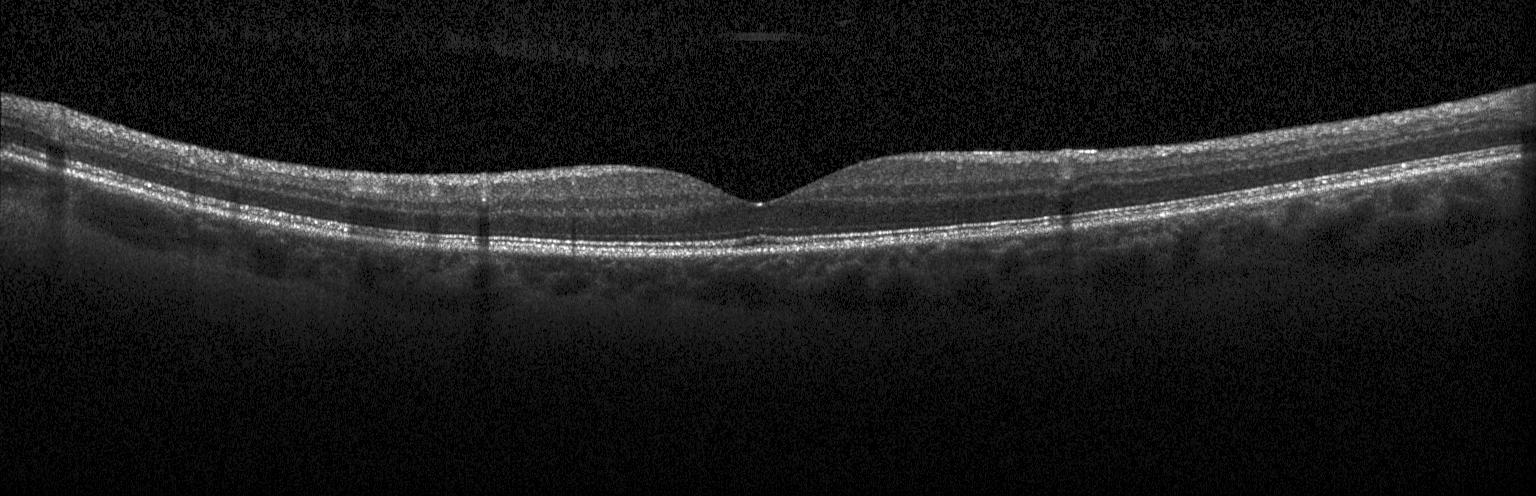
Optical coherence tomography scan — Finding: no evidence of choroidal neovascularization, diabetic macular edema, or drusen.